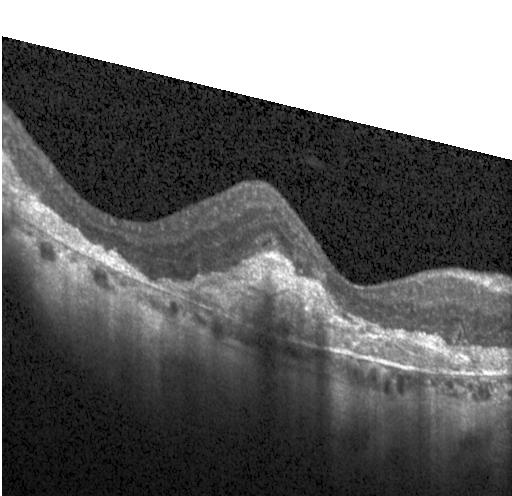
Dx: choroidal neovascularization (CNV).